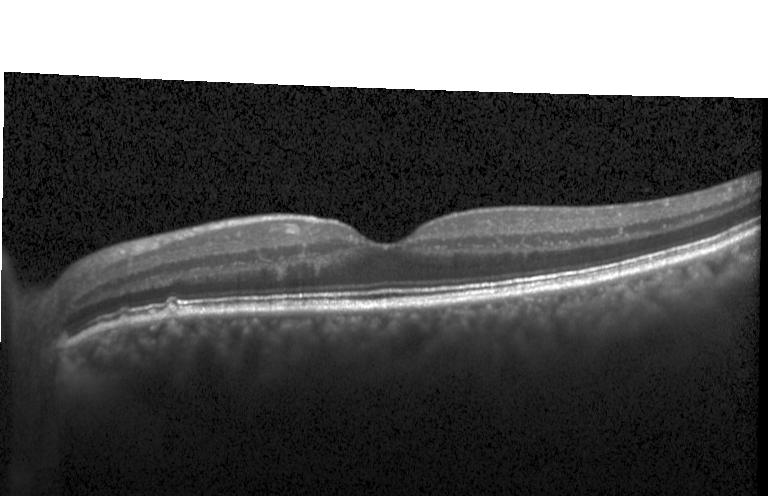 Instrument: Heidelberg Spectralis · optical coherence tomography scan · centered on the fovea. Impression: neither choroidal neovascularization, diabetic macular edema, nor drusen.